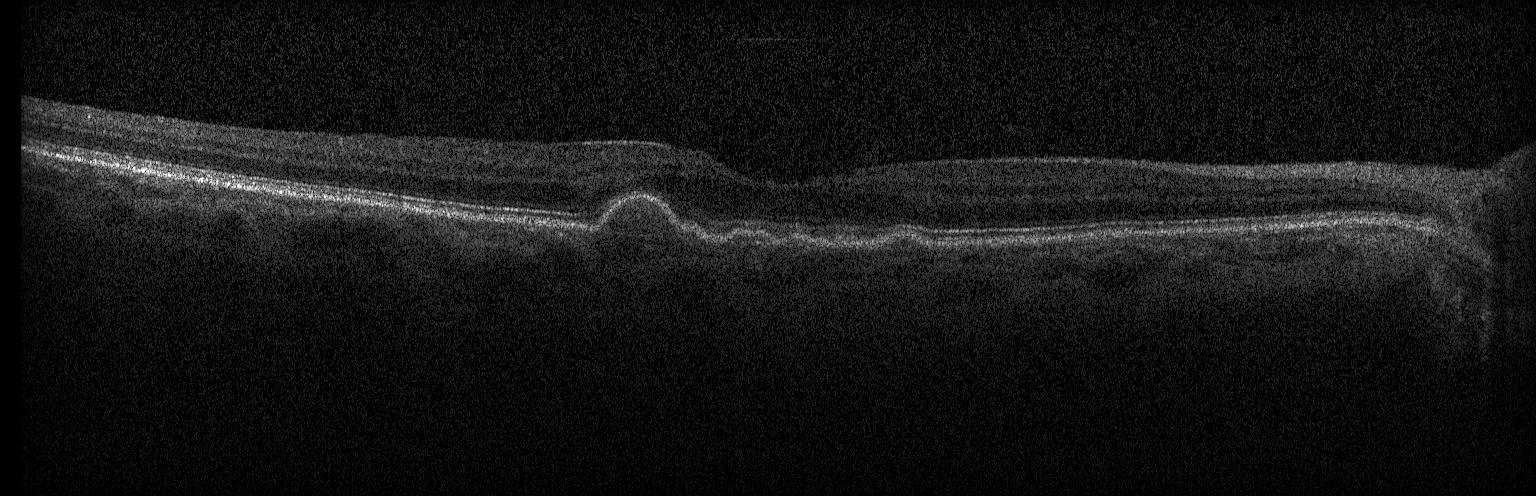

Impression: drusen.